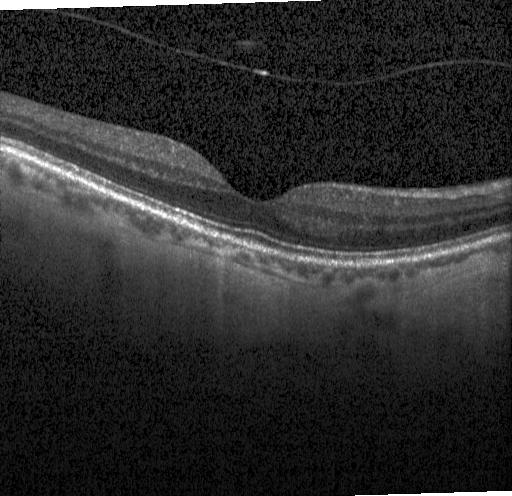
Macular OCT: neither choroidal neovascularization, diabetic macular edema, nor drusen.